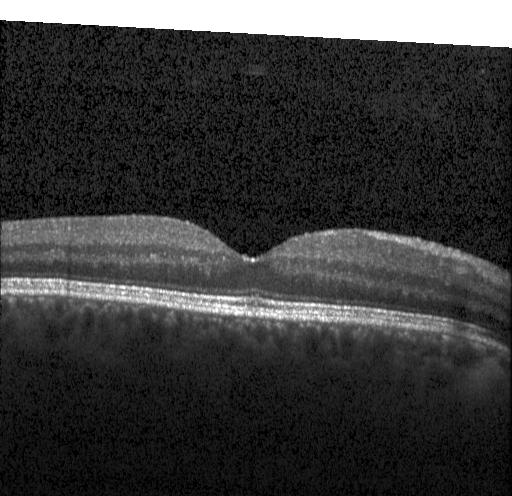
Spectral-domain optical coherence tomography. Through the macula. Retinal OCT B-scan. Impression: no evidence of choroidal neovascularization, diabetic macular edema, or drusen.